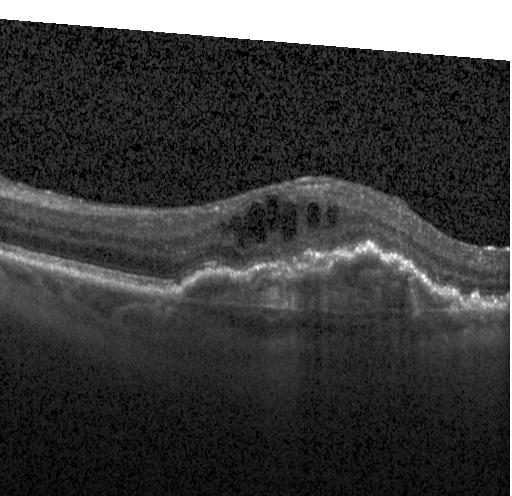 Retinal OCT B-scan — Finding: choroidal neovascularization.